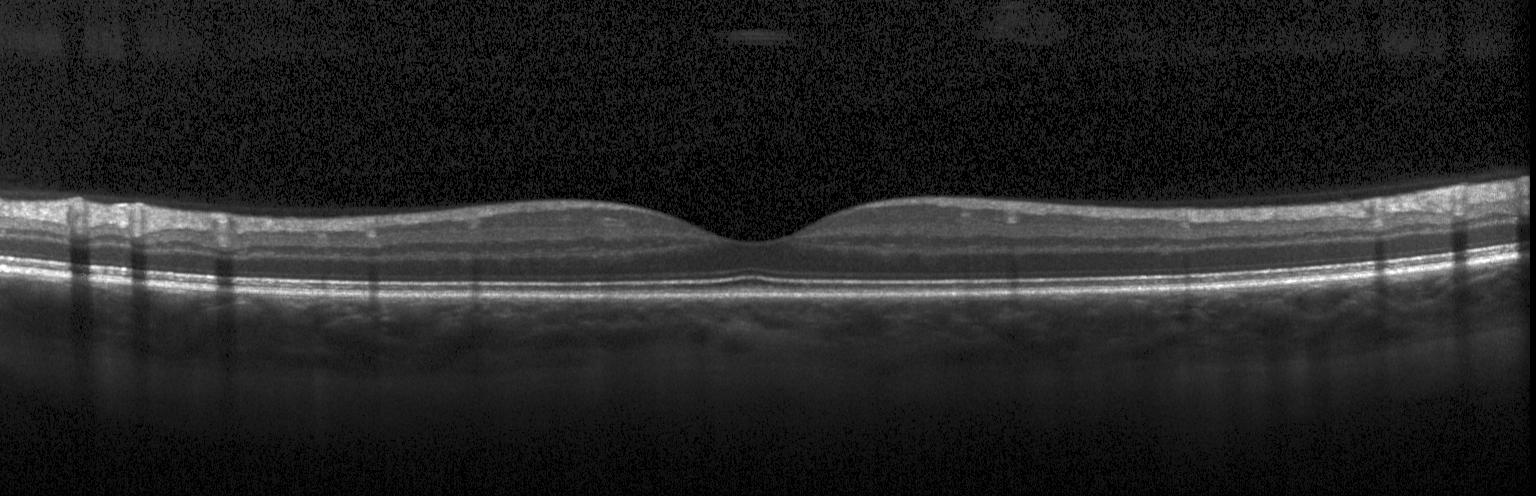

Spectral-domain OCT, Heidelberg Spectralis OCT system, optical coherence tomography scan. Macular OCT: no evidence of choroidal neovascularization, diabetic macular edema, or drusen.